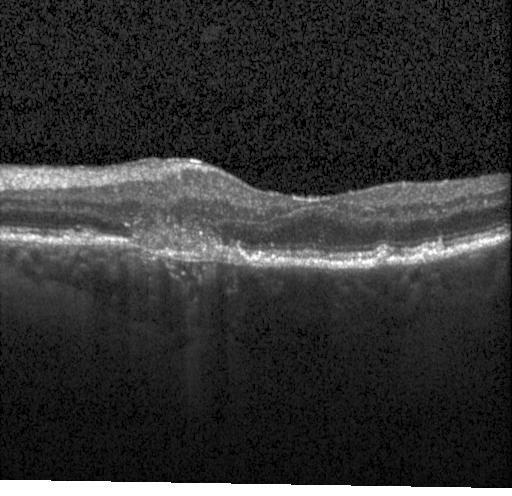 Optical coherence tomography scan — Assessment: CNV.